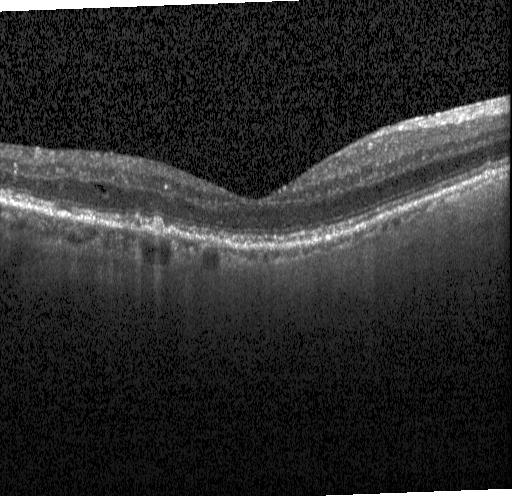
Heidelberg Spectralis · spectral-domain OCT · retinal OCT cross-section · horizontal scan through the fovea. The scan shows sub-RPE drusenoid deposits.